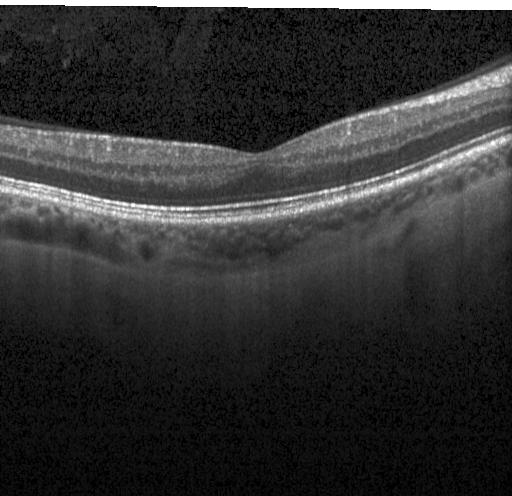 Macular OCT demonstrating neither choroidal neovascularization, diabetic macular edema, nor drusen.